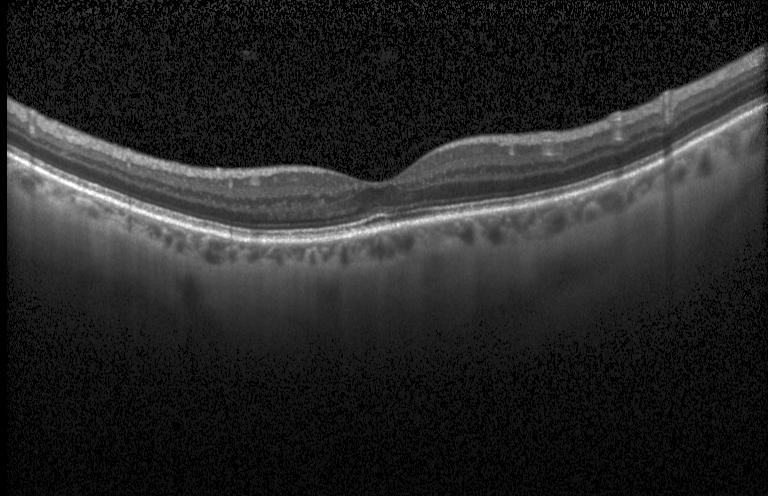

OCT B-scan showing no evidence of choroidal neovascularization, diabetic macular edema, or drusen.